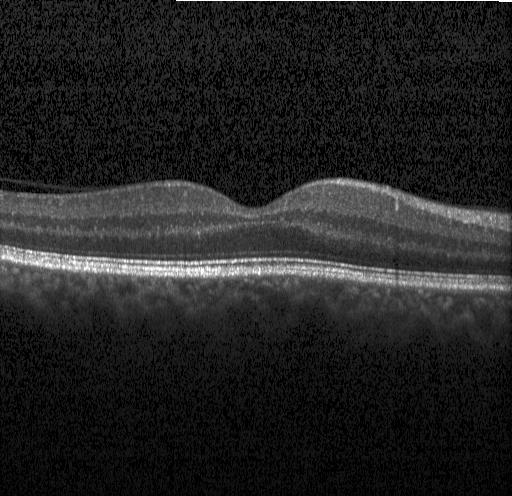

Optical coherence tomography scan; Heidelberg Spectralis OCT system; spectral-domain optical coherence tomography; macular scan
Macular OCT: no CNV, DME, or drusen.